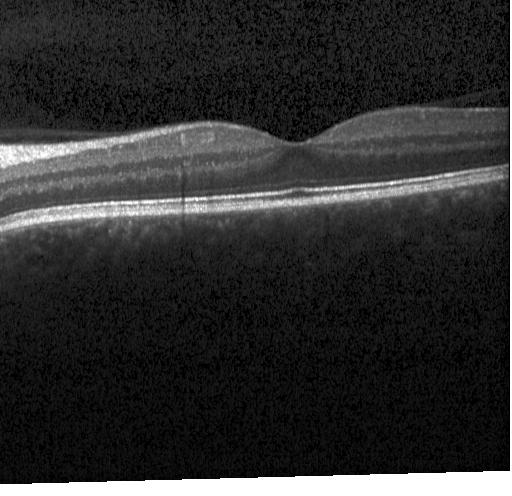 OCT line scan
This B-scan demonstrates no CNV, DME, or drusen.